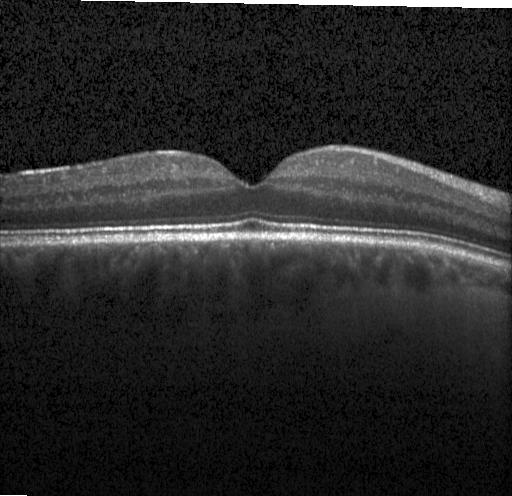 Diagnosis: no evidence of choroidal neovascularization, diabetic macular edema, or drusen.